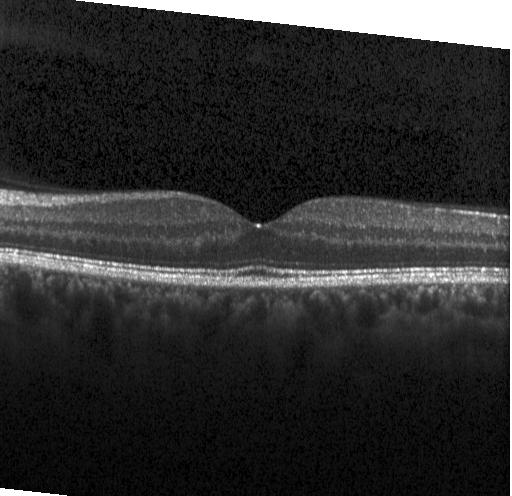

Heidelberg Spectralis OCT system; macular scan; optical coherence tomography B-scan. Impression: neither choroidal neovascularization, diabetic macular edema, nor drusen.